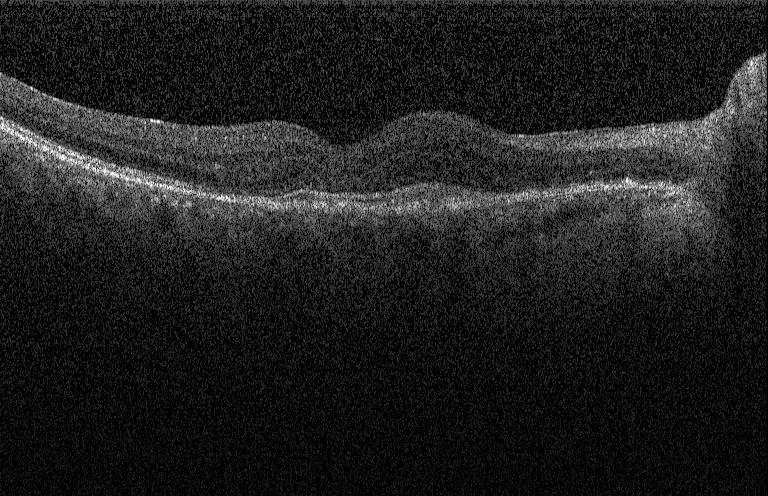

Optical coherence tomography B-scan · Heidelberg Spectralis · spectral-domain optical coherence tomography — Assessment: a choroidal neovascular membrane.